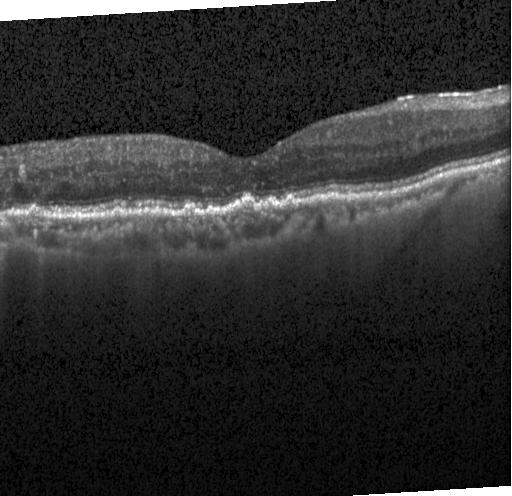
Heidelberg Spectralis OCT system · retinal OCT B-scan · SD-OCT · centered on the fovea.
Dx: sub-RPE drusenoid deposits.